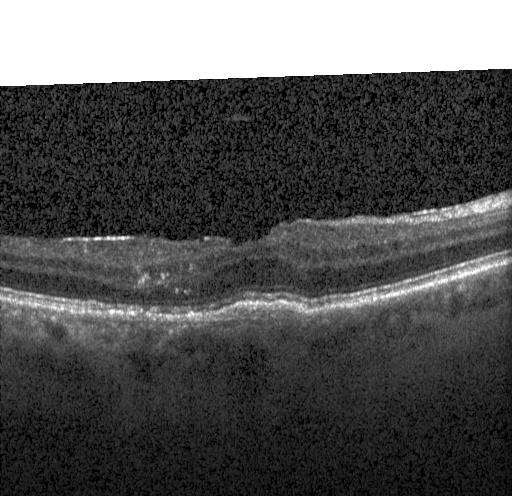 Optical coherence tomography B-scan · centered on the fovea.
Dx: choroidal neovascularization.